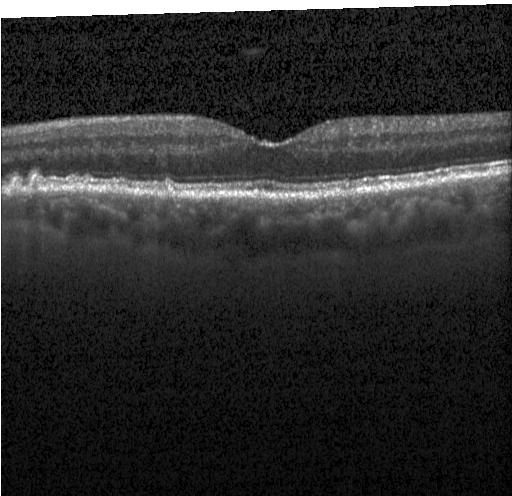
Macular scan; OCT line scan; spectral-domain OCT — This B-scan demonstrates multiple drusen.